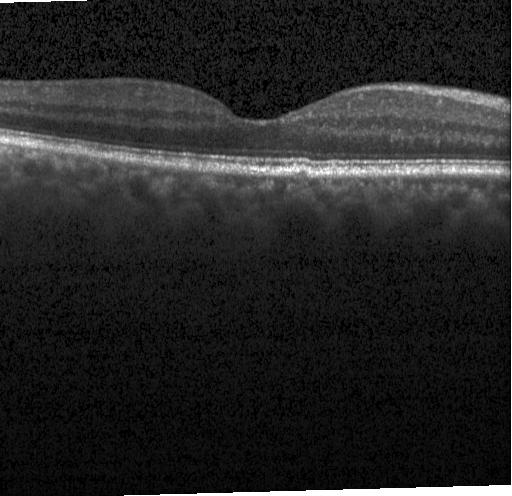

Assessment: no choroidal neovascularization, no diabetic macular edema, and no drusen.